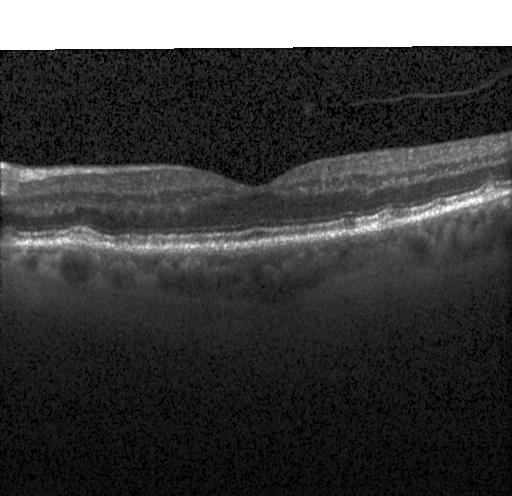
OCT B-scan. Impression: sub-RPE drusenoid deposits.